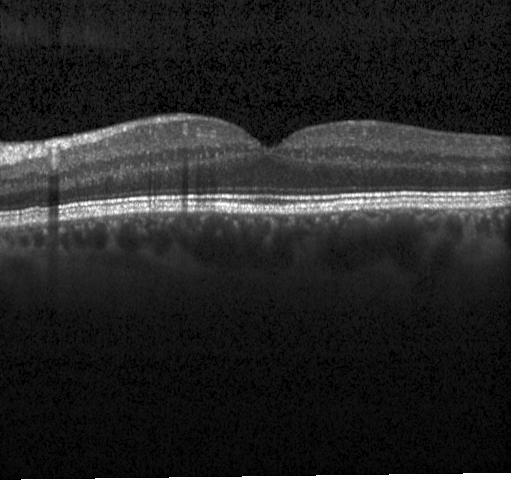 Retinal OCT B-scan, through the macula, Heidelberg Spectralis
Finding: neither CNV, DME, nor drusen.